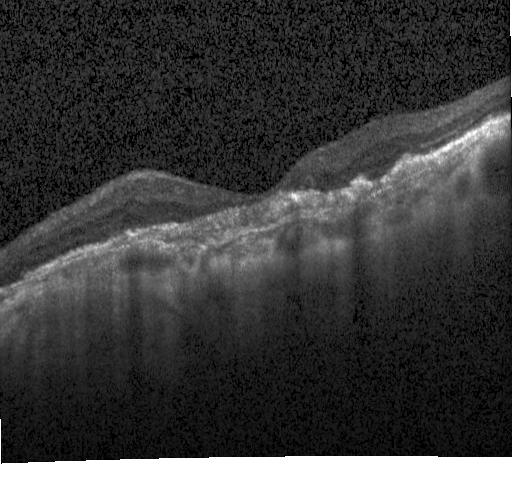 Optical coherence tomography B-scan.
The scan shows a choroidal neovascular membrane.